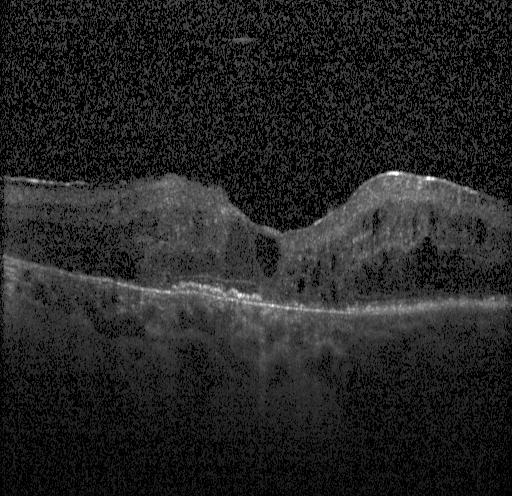 OCT B-scan
Finding: a choroidal neovascular membrane.